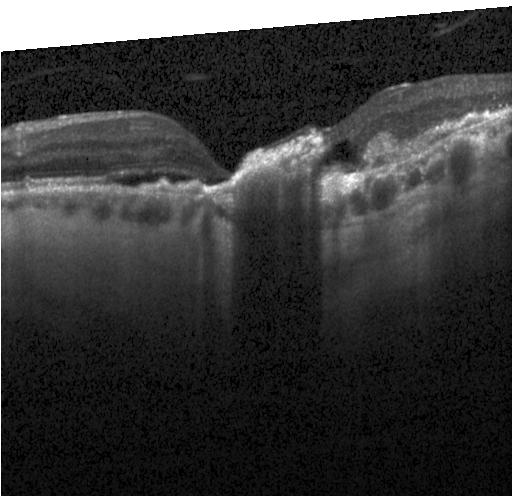 Heidelberg Spectralis · retinal OCT B-scan — Assessment: CNV.